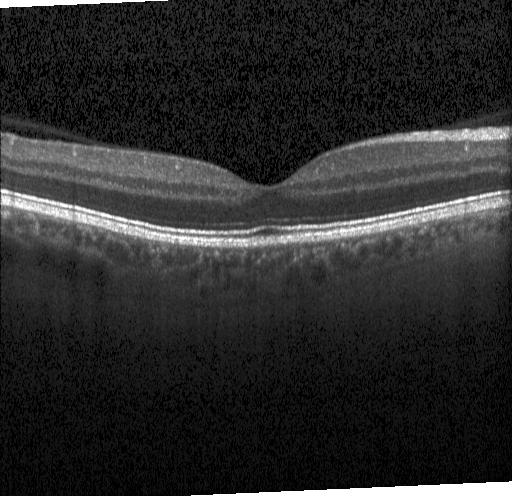 This B-scan demonstrates neither choroidal neovascularization, diabetic macular edema, nor drusen.